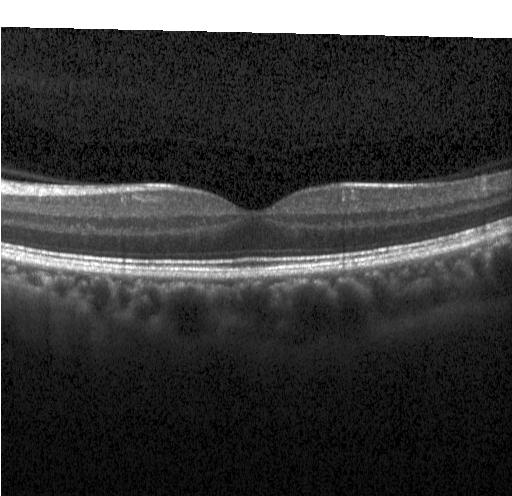

Dx: no choroidal neovascularization, diabetic macular edema, or drusen.